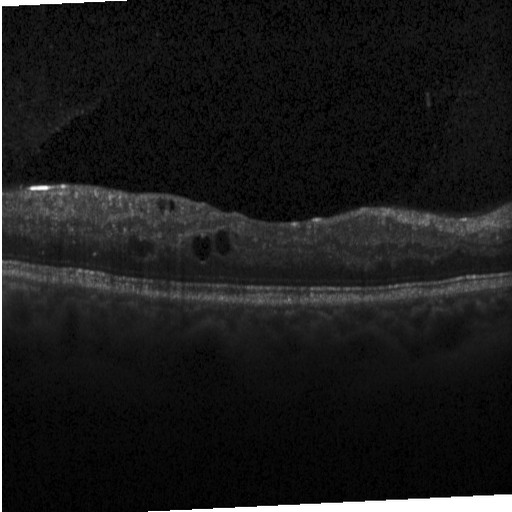
OCT line scan, Heidelberg Spectralis. Impression: diabetic macular edema.